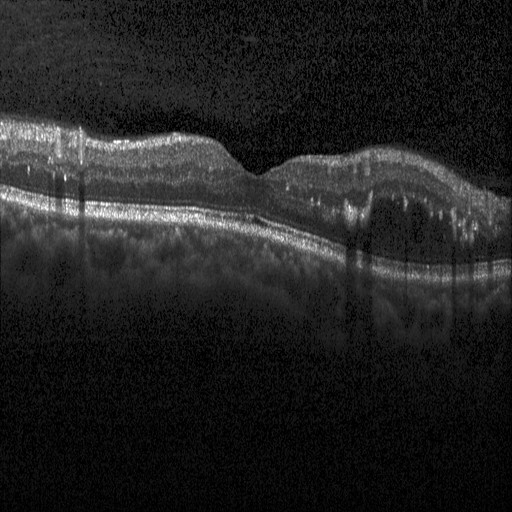
Optical coherence tomography scan — OCT finding: diabetic macular edema (DME).